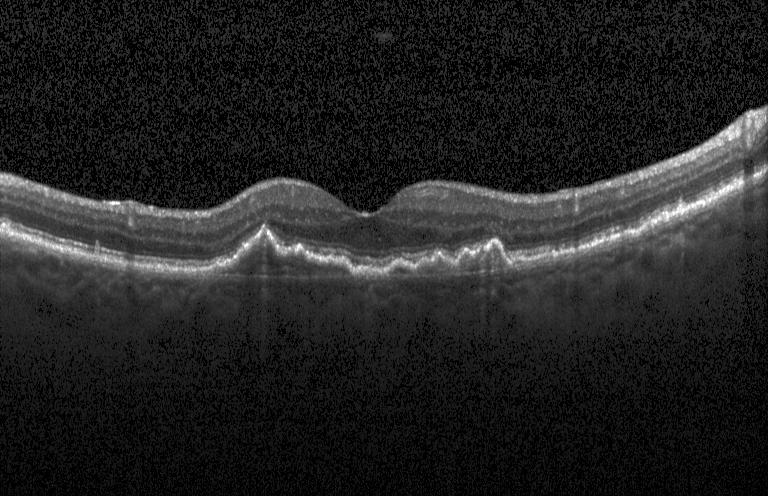 The scan shows choroidal neovascularization (CNV).